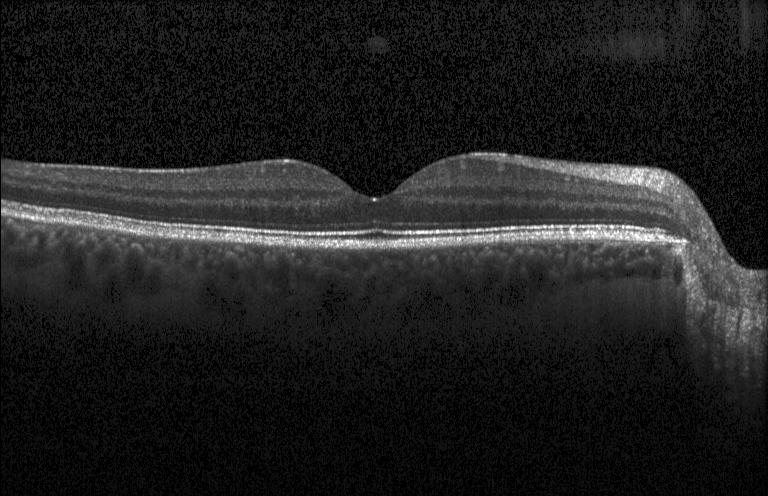 Optical coherence tomography B-scan
Finding: no choroidal neovascularization, diabetic macular edema, or drusen.